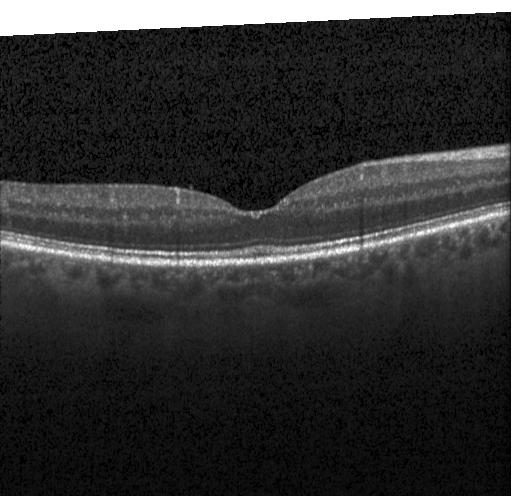
Retinal OCT B-scan. Finding: no CNV, no DME, and no drusen.